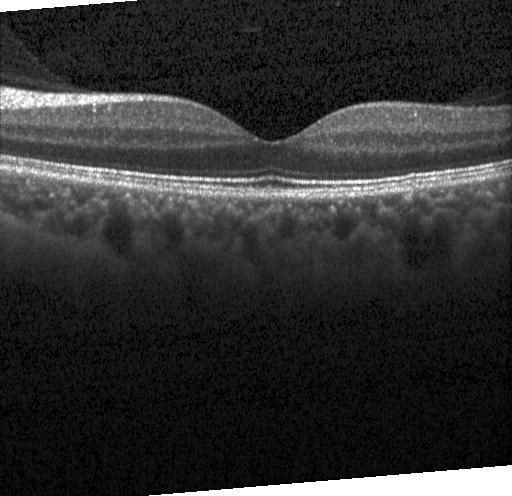

Spectral-domain optical coherence tomography; Heidelberg Spectralis OCT system; centered on the fovea; retinal OCT cross-section.
Diagnosis: no CNV, DME, or drusen.